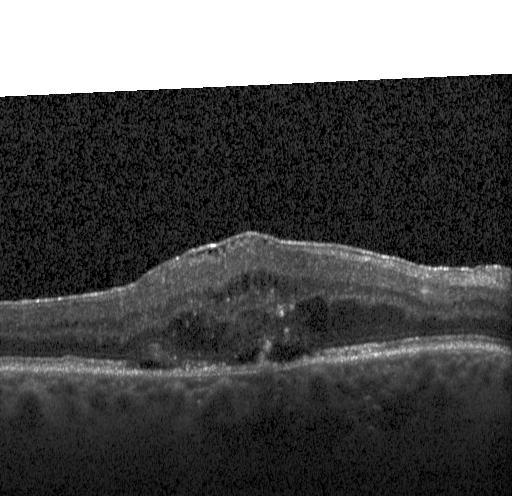

OCT B-scan. Diagnosis: CNV.